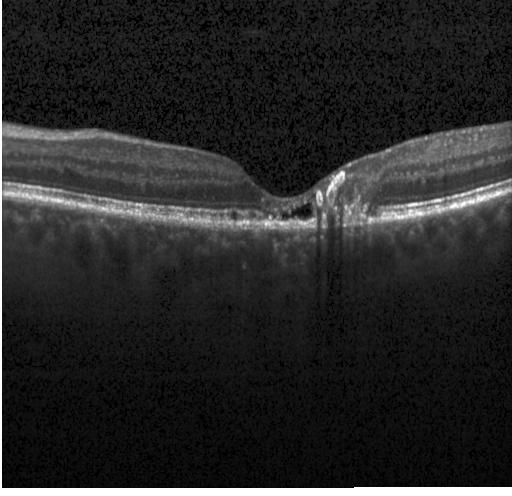

Horizontal scan through the fovea, optical coherence tomography B-scan, Heidelberg Spectralis OCT system, spectral-domain optical coherence tomography
A choroidal neovascular membrane.